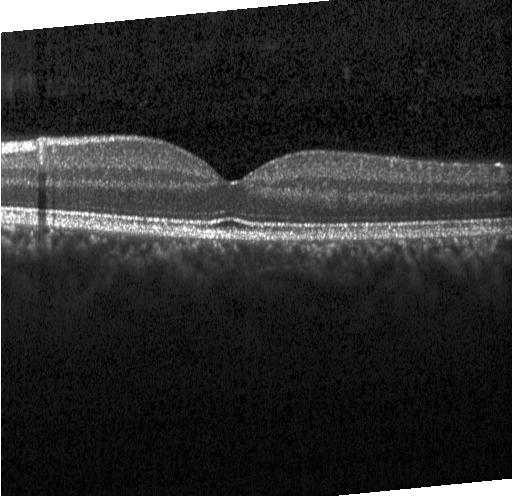 Spectral-domain OCT B-scan: no choroidal neovascularization, diabetic macular edema, or drusen.